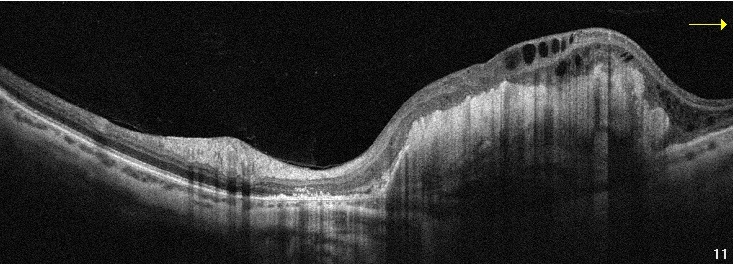
Retinal OCT cross-section.
Dx: age-related macular degeneration.